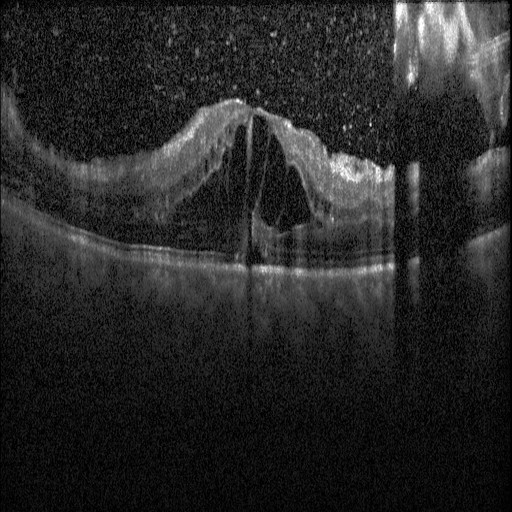
Heidelberg Spectralis; retinal OCT B-scan; spectral-domain optical coherence tomography; centered on the fovea
Impression: diabetic macular edema (DME).